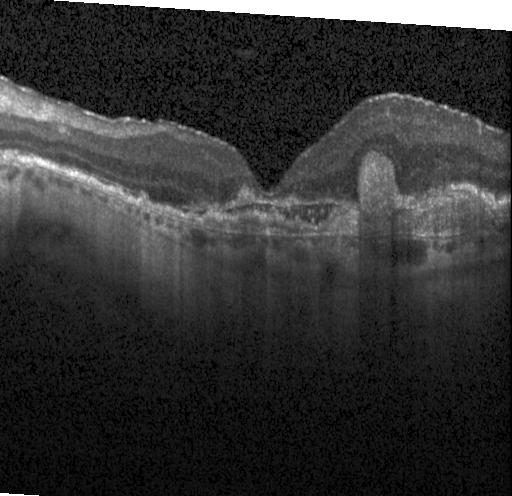 Dx: a choroidal neovascular membrane.